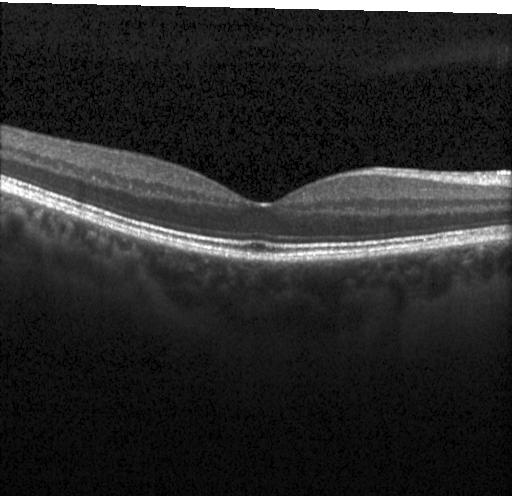

Diagnosis: no CNV, DME, or drusen.